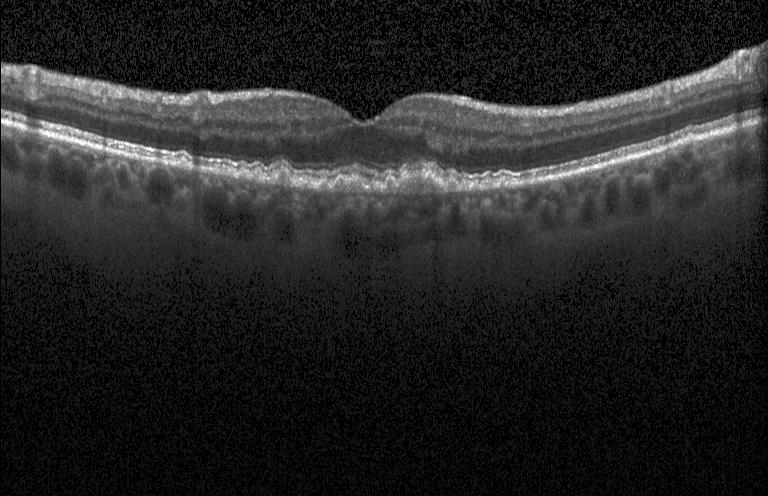

This B-scan demonstrates sub-RPE drusenoid deposits.